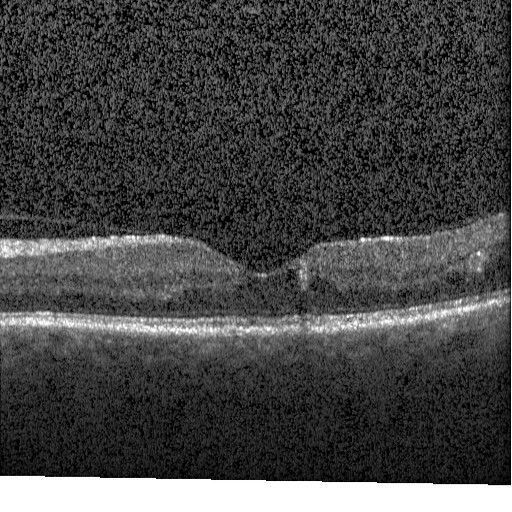
The scan shows diabetic macular edema.